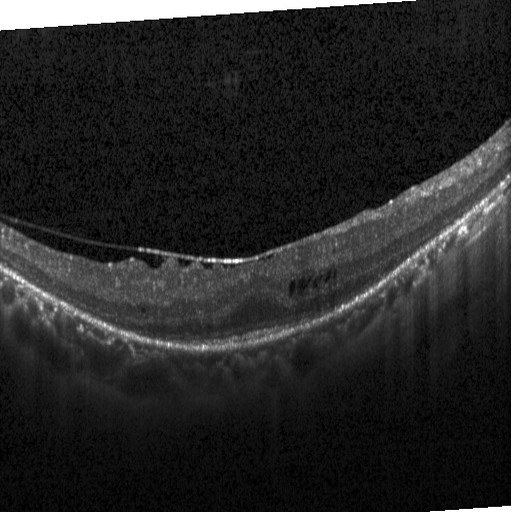 Impression: DME.